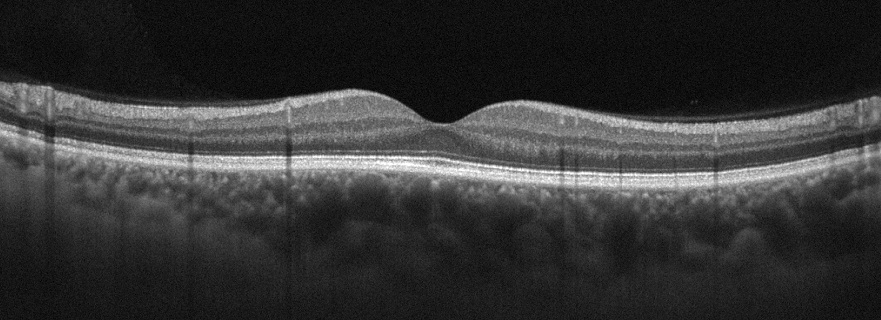

Retinal OCT cross-section
Impression: no AMD, DME, ERM, RAO, RVO, or VID.